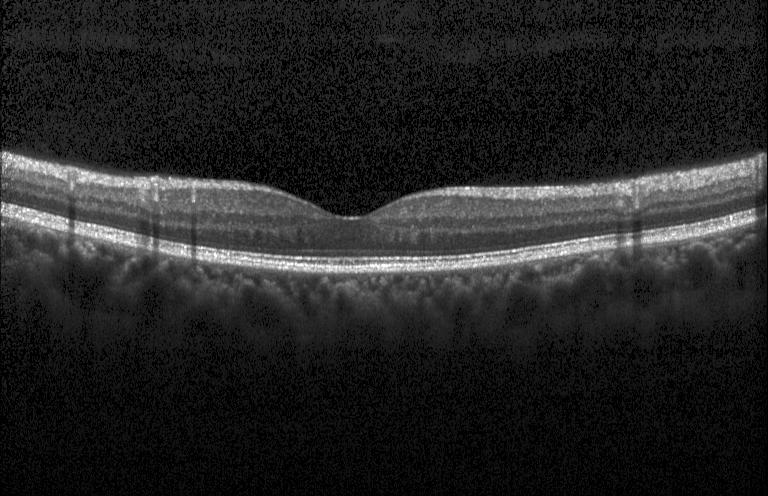 This B-scan demonstrates neither CNV, DME, nor drusen.